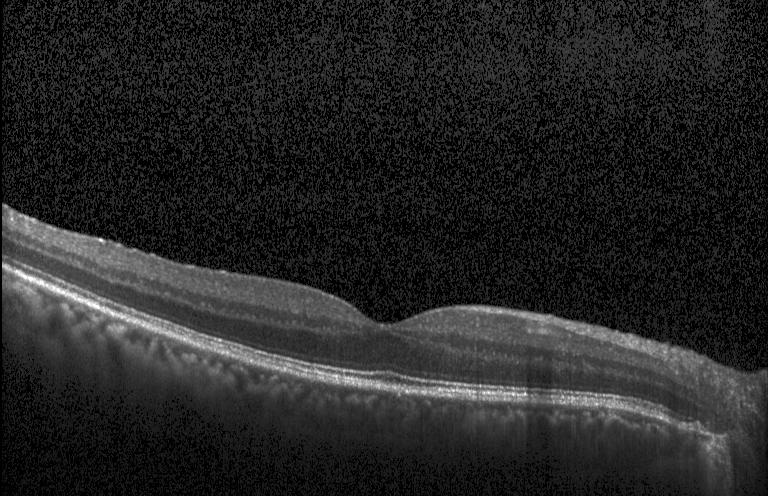 OCT B-scan · SD-OCT. This B-scan demonstrates neither choroidal neovascularization, diabetic macular edema, nor drusen.